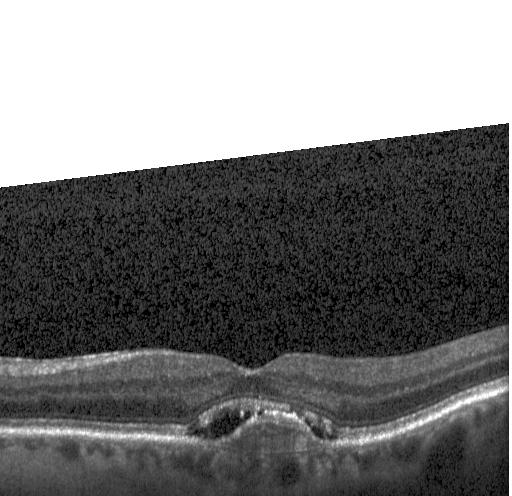
Optical coherence tomography scan. Heidelberg Spectralis — OCT finding: a choroidal neovascular membrane.